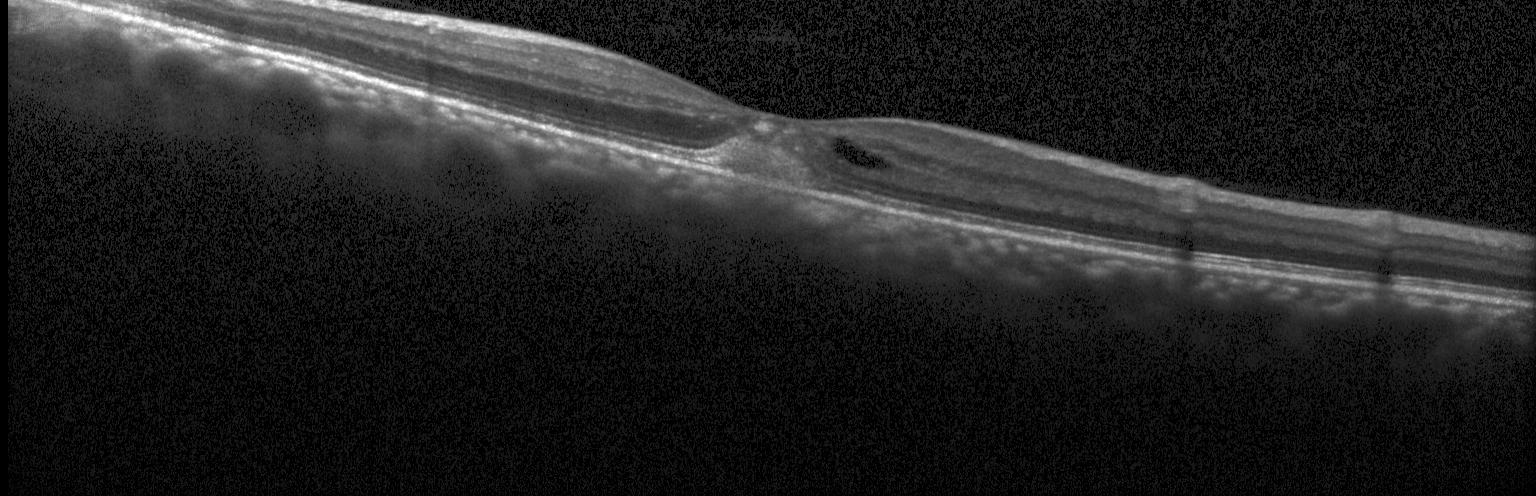

Impression: CNV.